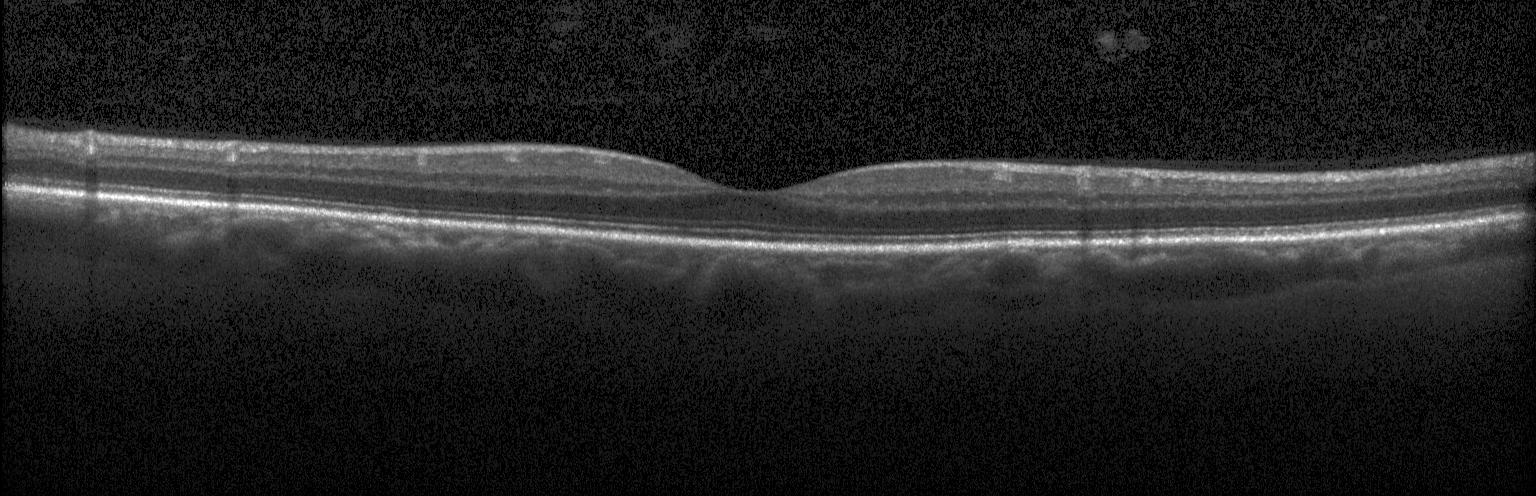

Optical coherence tomography B-scan — OCT finding: no evidence of CNV, DME, or drusen.